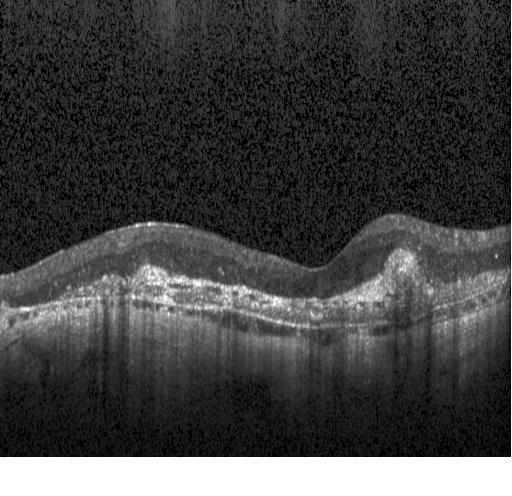 Finding: a choroidal neovascular membrane.